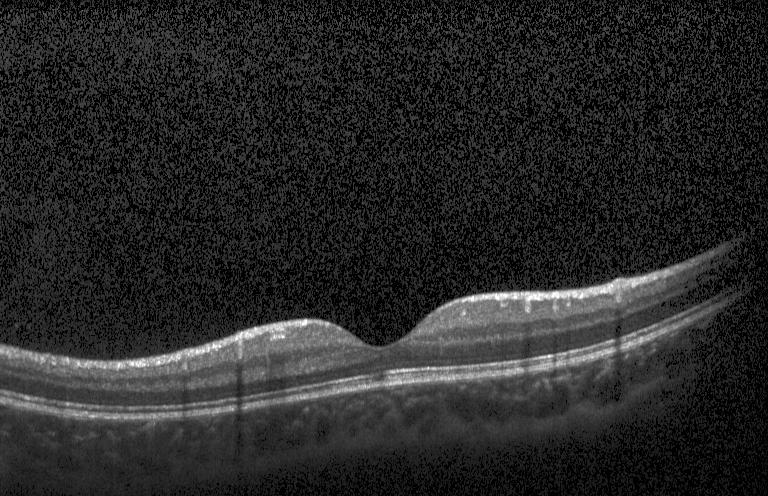
Instrument: Heidelberg Spectralis · optical coherence tomography B-scan
Macular OCT: no CNV, DME, or drusen.